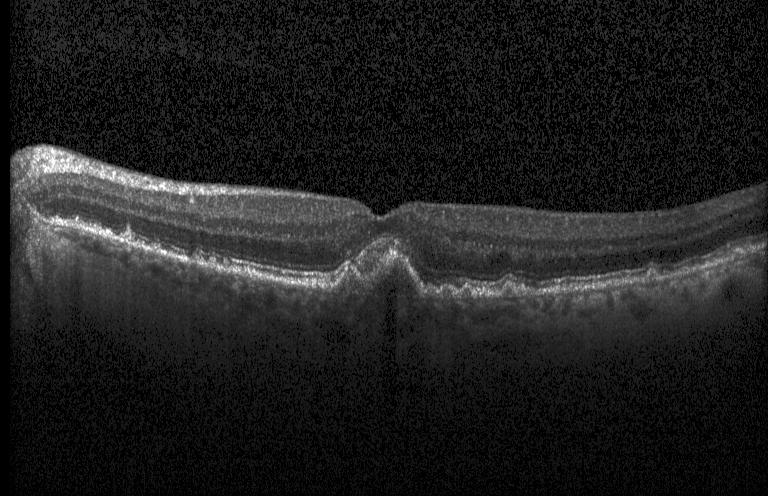
Fovea-centered. Retinal OCT cross-section. Heidelberg Spectralis OCT system. Finding: choroidal neovascularization (CNV).